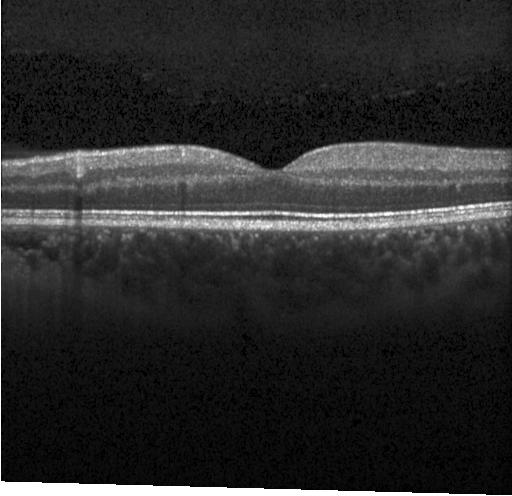 Diagnosis: no CNV, no DME, and no drusen.